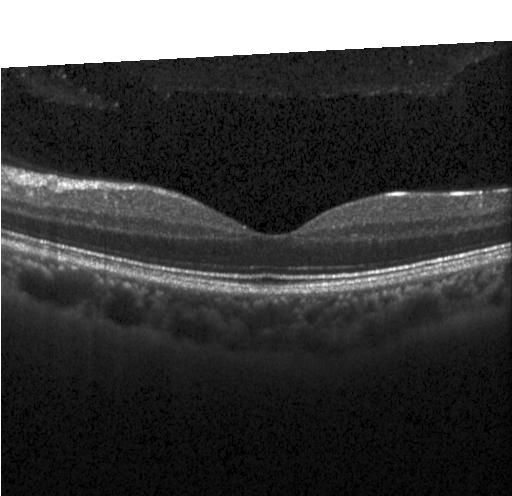

OCT B-scan. No CNV, DME, or drusen.